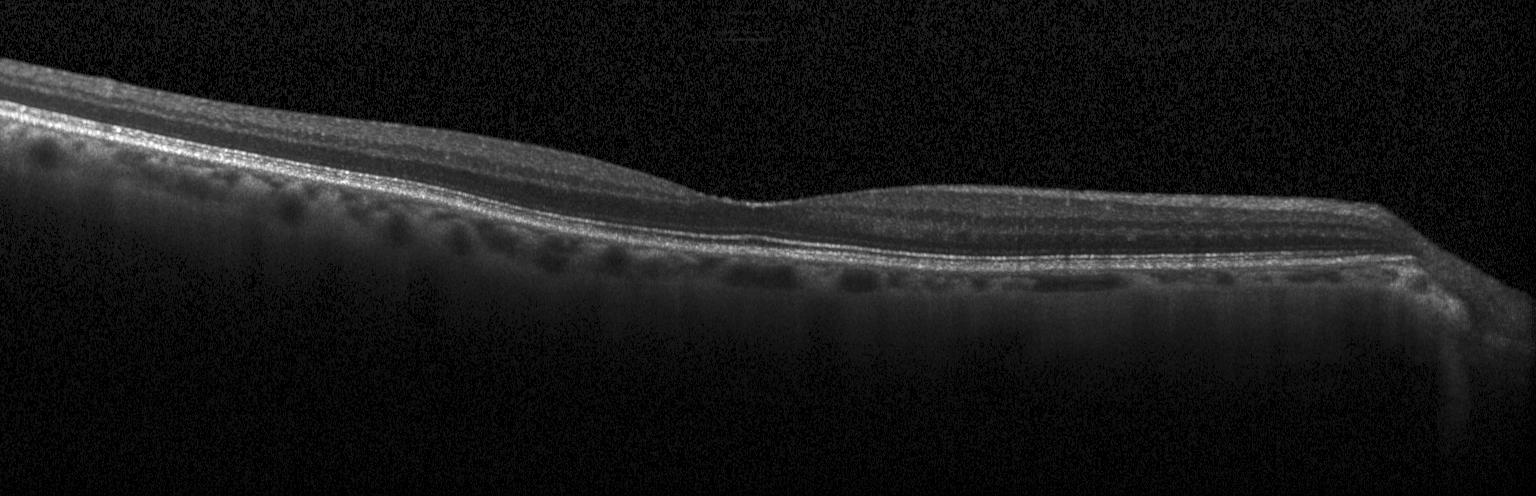

This B-scan demonstrates neither choroidal neovascularization, diabetic macular edema, nor drusen.